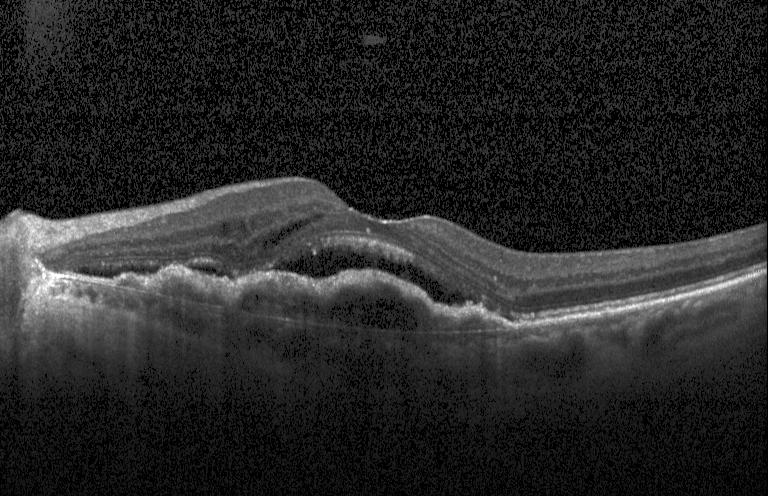

Finding: choroidal neovascularization (CNV).